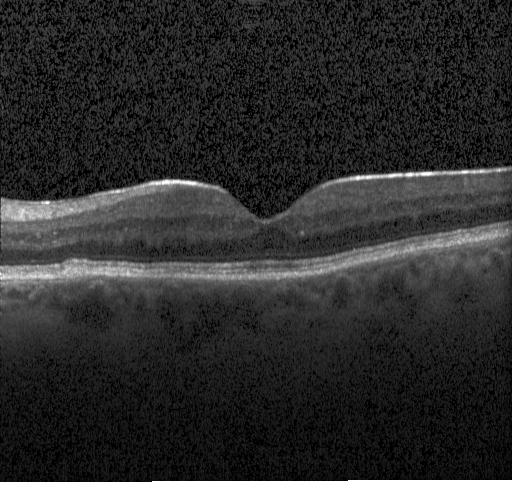

Retinal OCT cross-section, spectral-domain optical coherence tomography, Heidelberg Spectralis.
Impression: no choroidal neovascularization, diabetic macular edema, or drusen.